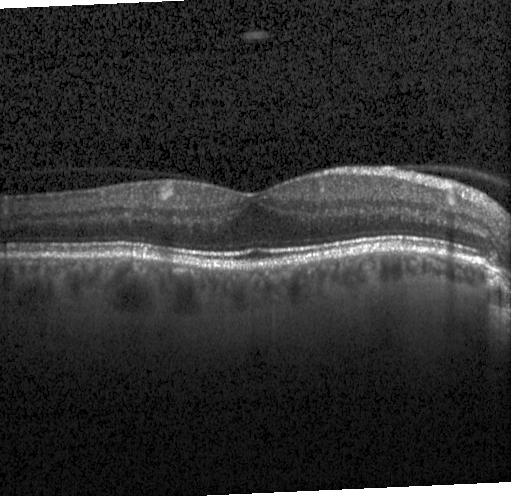
Retinal OCT B-scan. Through the macula. Spectral-domain OCT. Finding: neither choroidal neovascularization, diabetic macular edema, nor drusen.